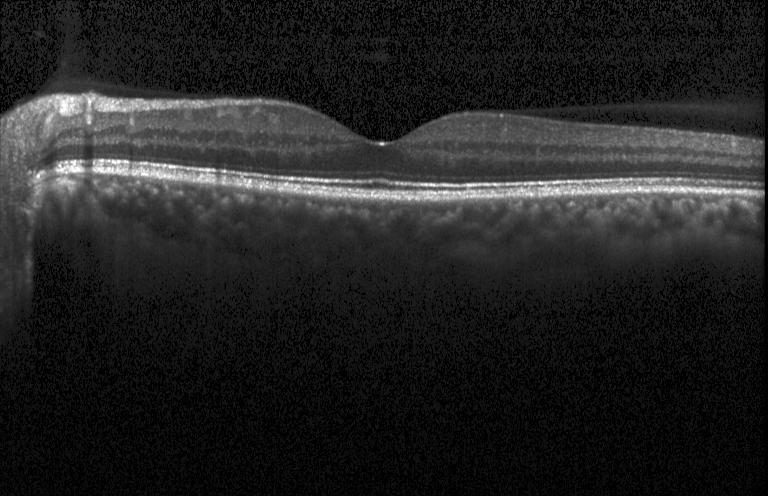
Finding: no choroidal neovascularization, no diabetic macular edema, and no drusen.